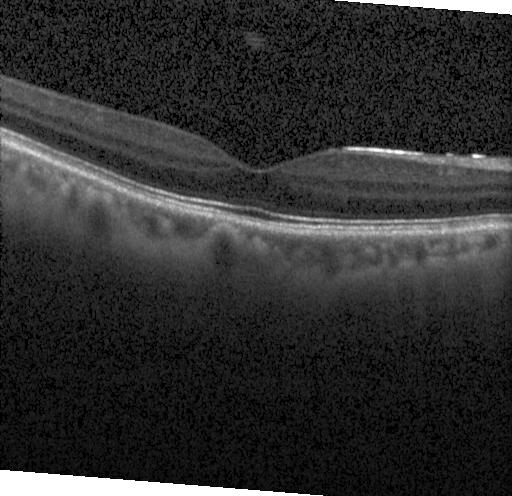

Macular scan · optical coherence tomography scan. Diagnosis: no evidence of choroidal neovascularization, diabetic macular edema, or drusen.